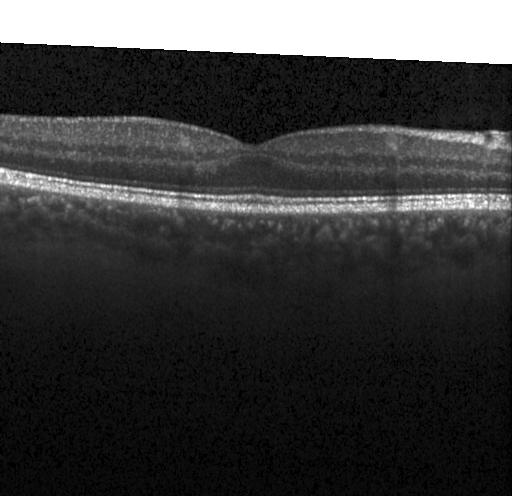

Retinal OCT B-scan.
Dx: no choroidal neovascularization, diabetic macular edema, or drusen.